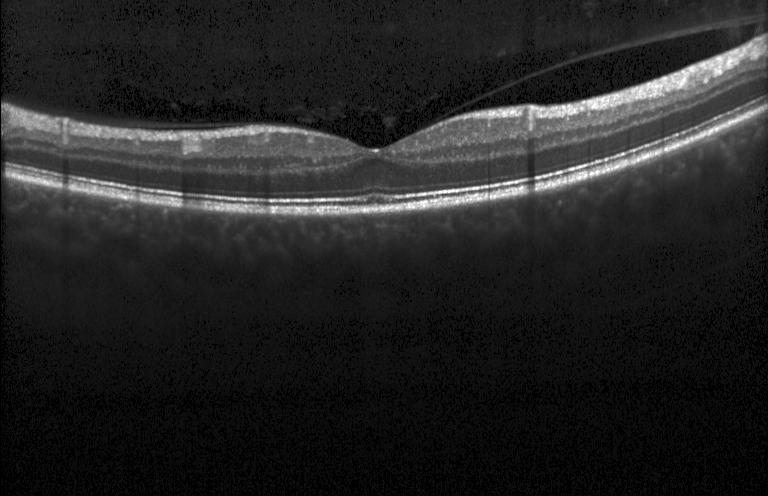 SD-OCT. Fovea-centered. Optical coherence tomography scan
This B-scan demonstrates no choroidal neovascularization, no diabetic macular edema, and no drusen.